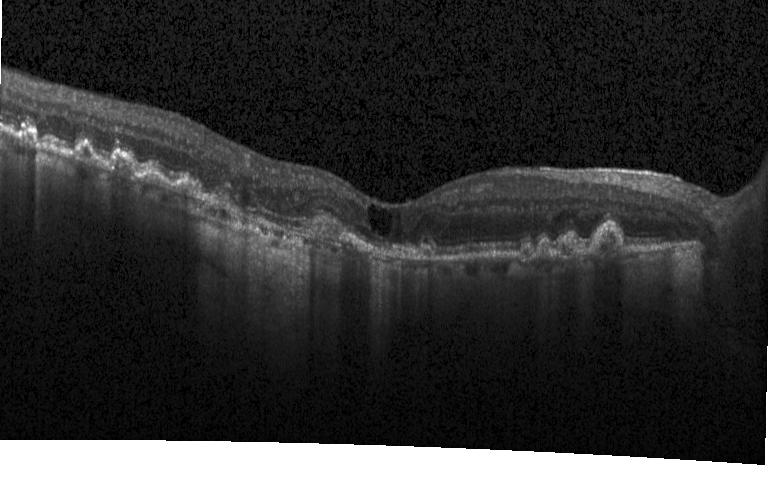 Retinal OCT B-scan
Assessment: a choroidal neovascular membrane.